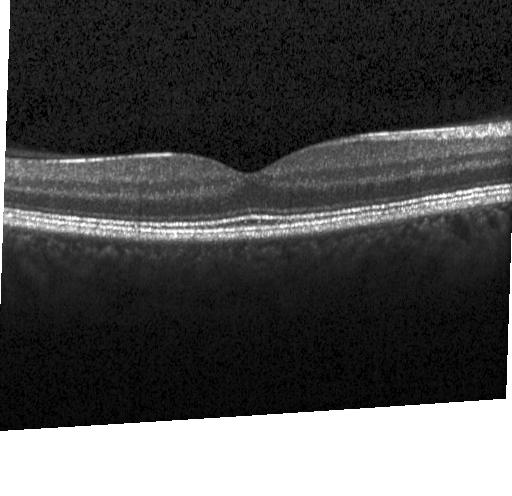

OCT finding: no evidence of choroidal neovascularization, diabetic macular edema, or drusen.